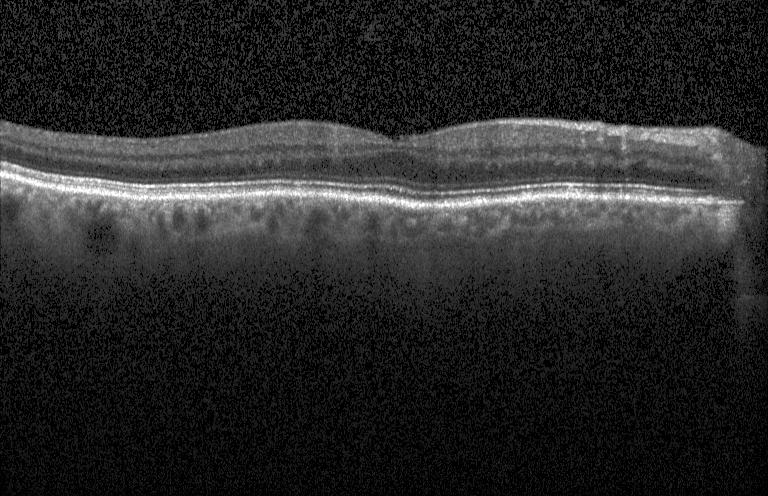

Retinal OCT B-scan · spectral-domain OCT · instrument: Heidelberg Spectralis · fovea-centered. Macular OCT: neither choroidal neovascularization, diabetic macular edema, nor drusen.